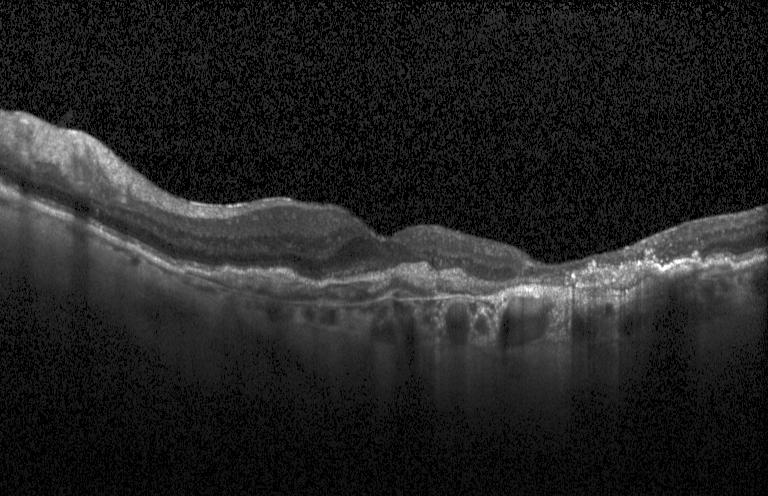

OCT B-scan; centered on the fovea — Dx: a choroidal neovascular membrane.